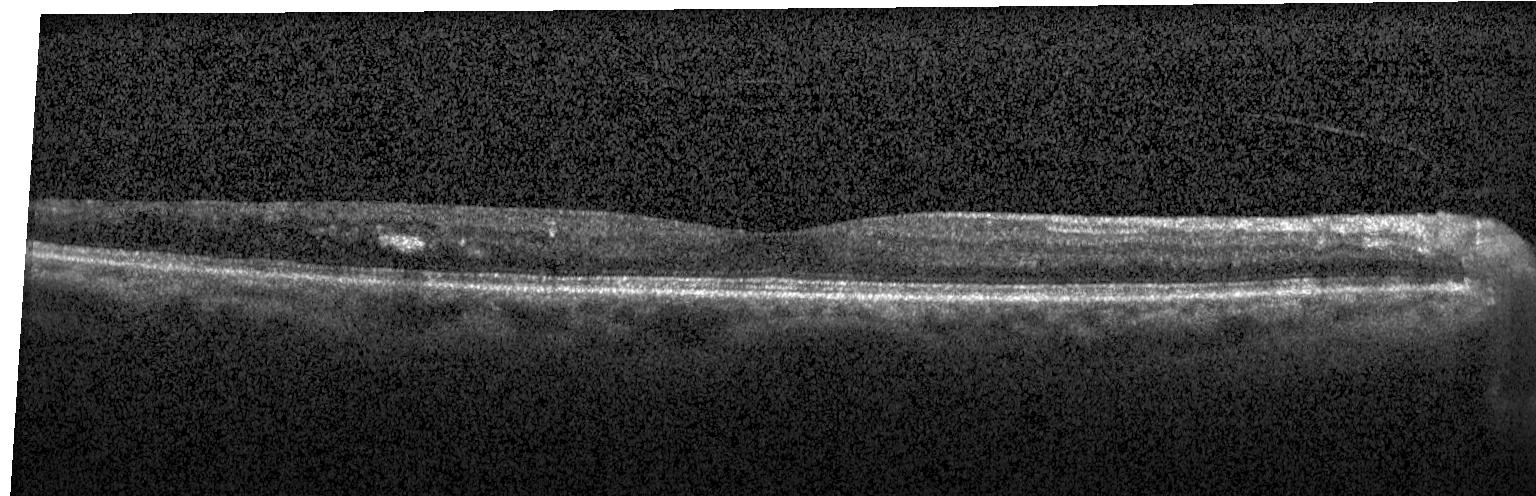 Macular OCT: diabetic macular edema (DME).